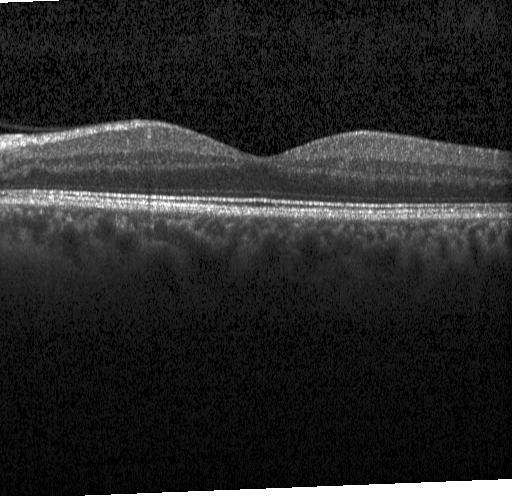
Spectral-domain OCT, optical coherence tomography B-scan, Heidelberg Spectralis — Diagnosis: no evidence of choroidal neovascularization, diabetic macular edema, or drusen.